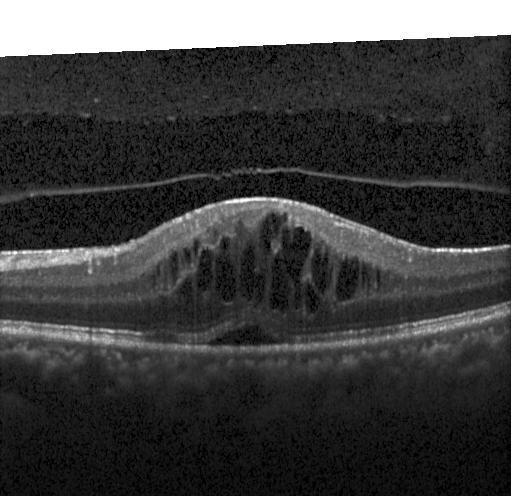

Retinal OCT cross-section
Assessment: DME.